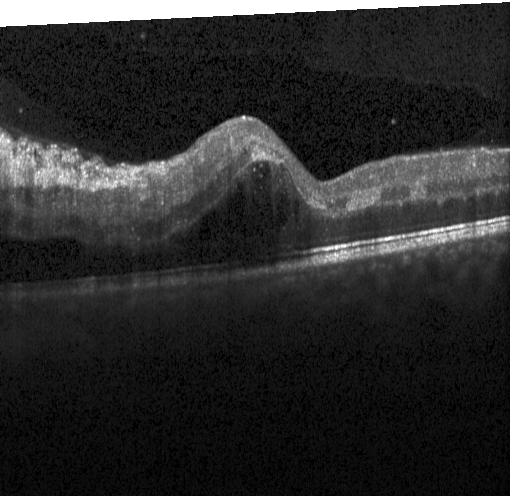 Through the macula; SD-OCT; retinal OCT B-scan
The scan shows diabetic macular edema (DME).